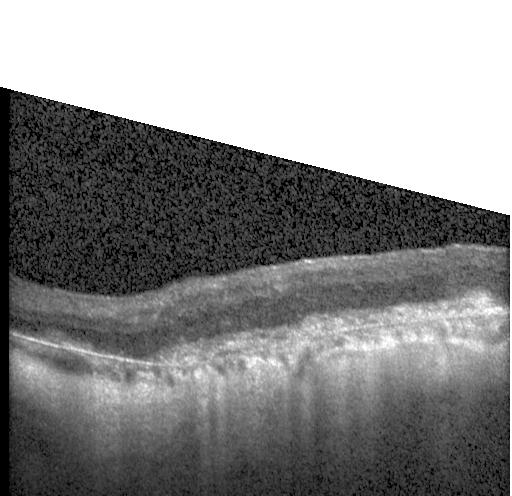 OCT scan showing CNV.